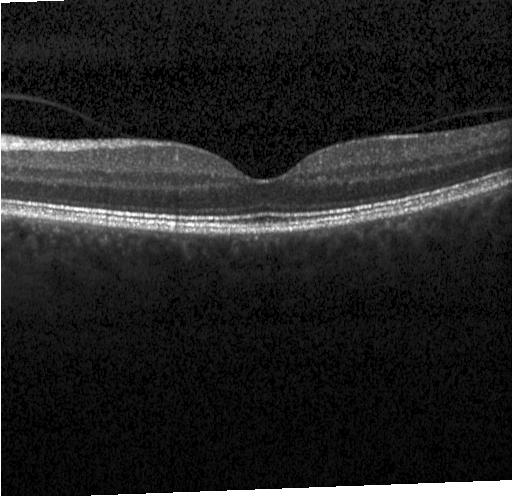
Spectral-domain OCT · optical coherence tomography scan
The scan shows no CNV, no DME, and no drusen.